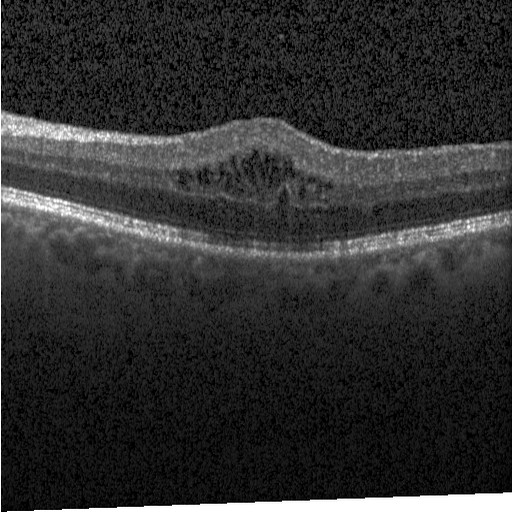
Acquired on a Heidelberg Spectralis, OCT line scan — Finding: DME.